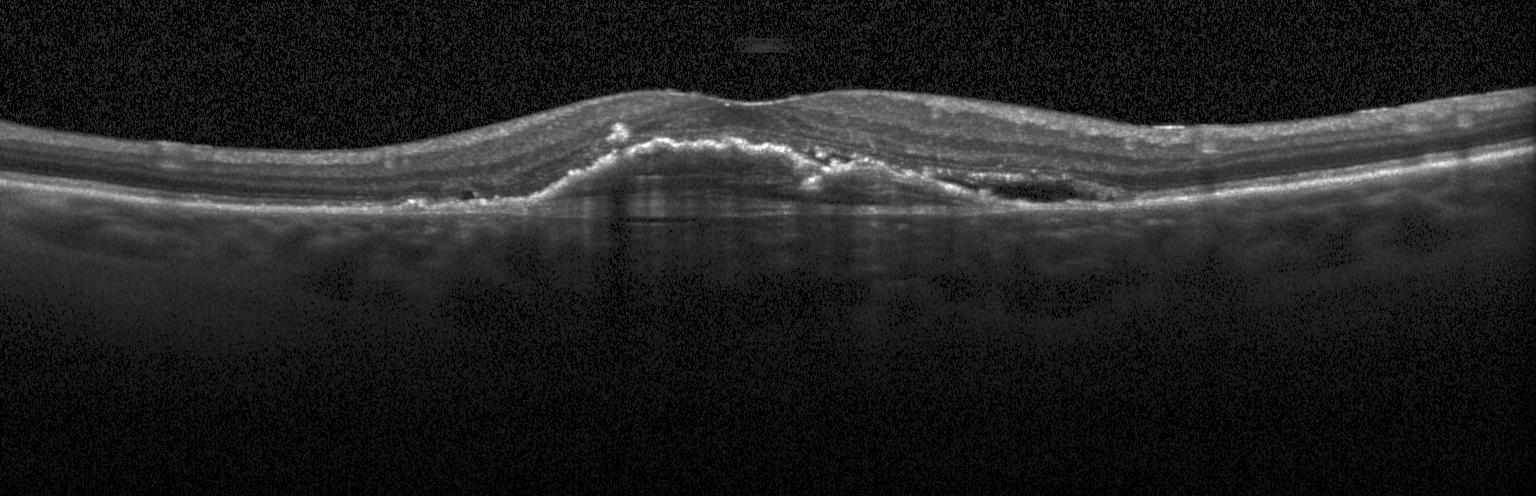
Macular scan, OCT B-scan, acquired on a Heidelberg Spectralis
This B-scan demonstrates a choroidal neovascular membrane.